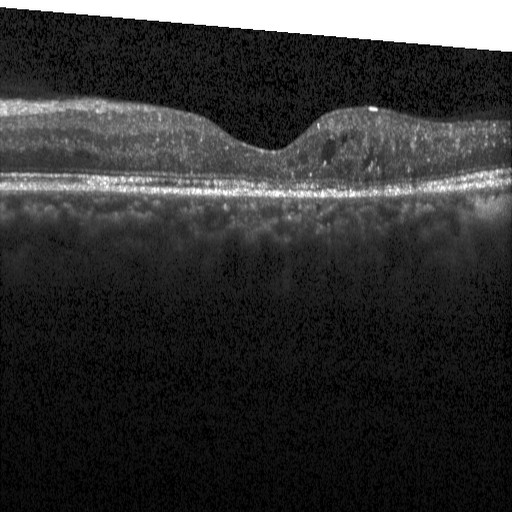

Retinal OCT B-scan. The scan shows diabetic macular edema (DME).